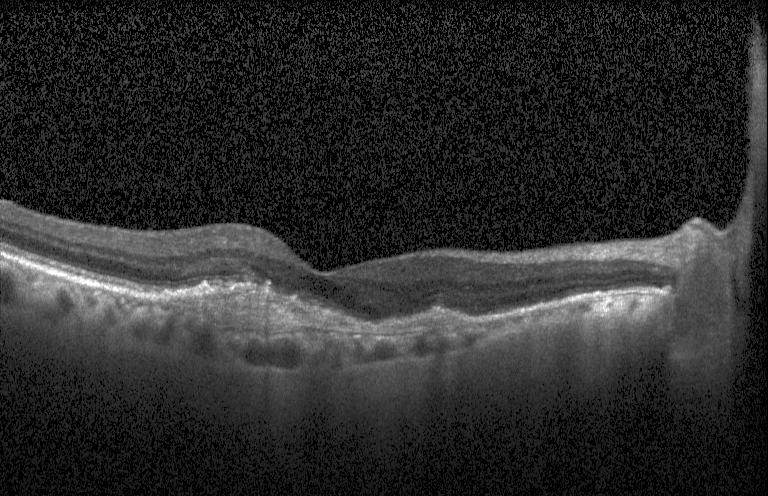 Assessment: a choroidal neovascular membrane.